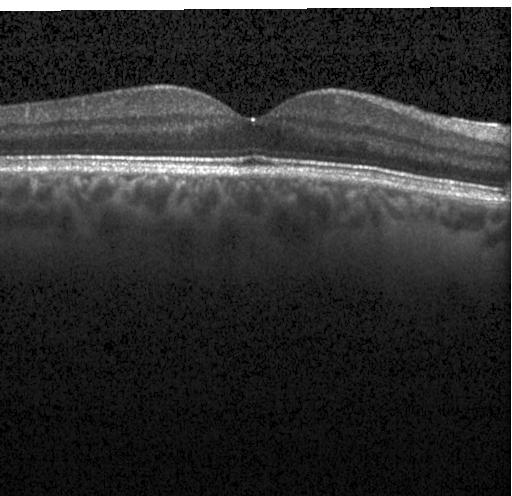 Optical coherence tomography scan. SD-OCT. Horizontal scan through the fovea. Impression: neither CNV, DME, nor drusen.